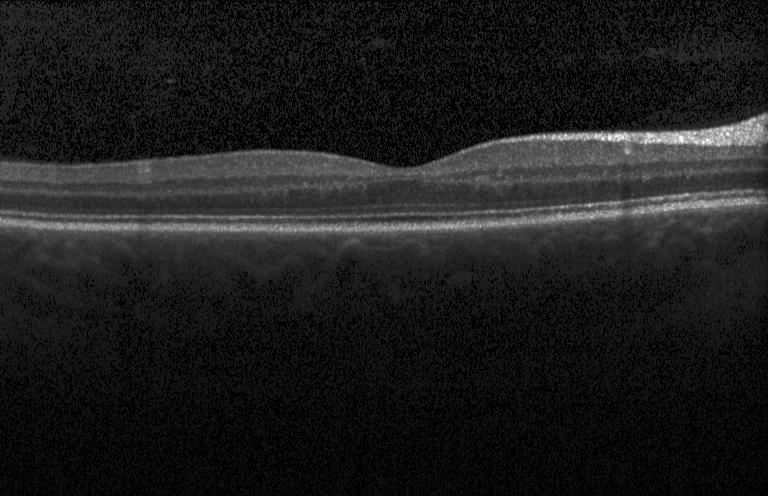
Horizontal scan through the fovea · retinal OCT cross-section
Impression: no evidence of choroidal neovascularization, diabetic macular edema, or drusen.